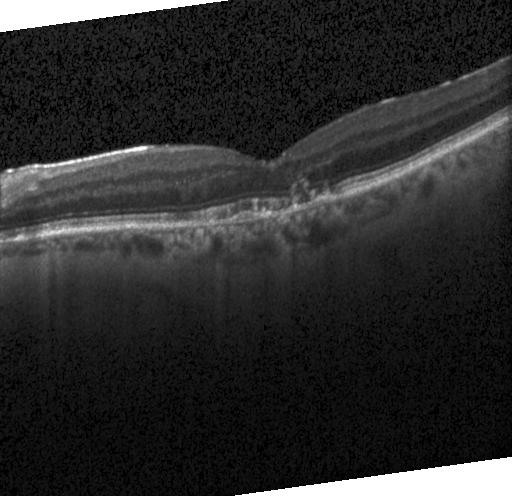
OCT scan showing a choroidal neovascular membrane.